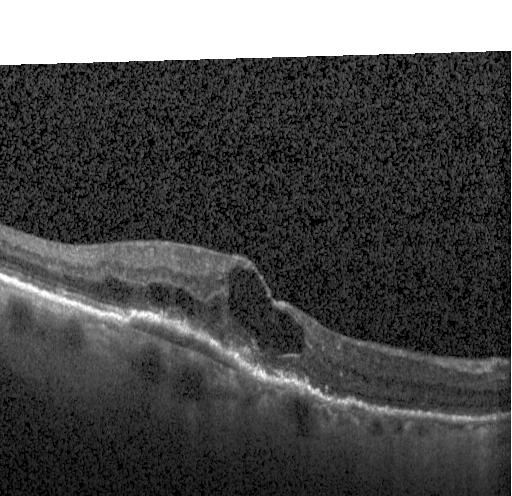
Impression: a choroidal neovascular membrane.